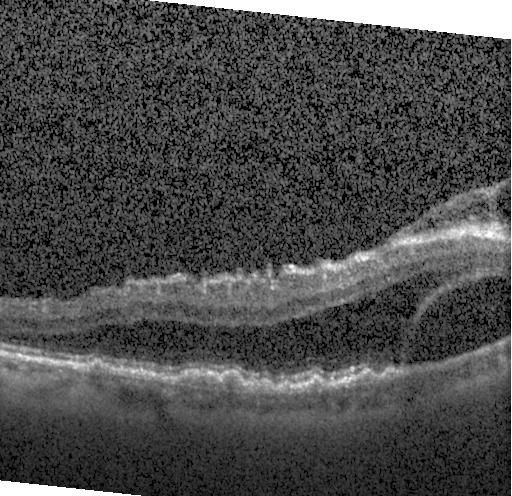
SD-OCT. Optical coherence tomography B-scan.
Macular OCT: choroidal neovascularization (CNV).